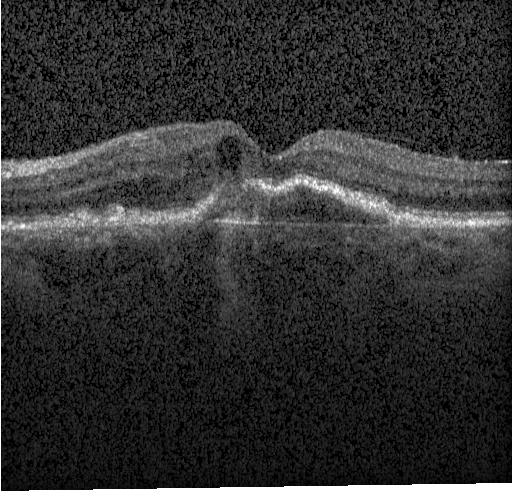
OCT B-scan showing CNV.